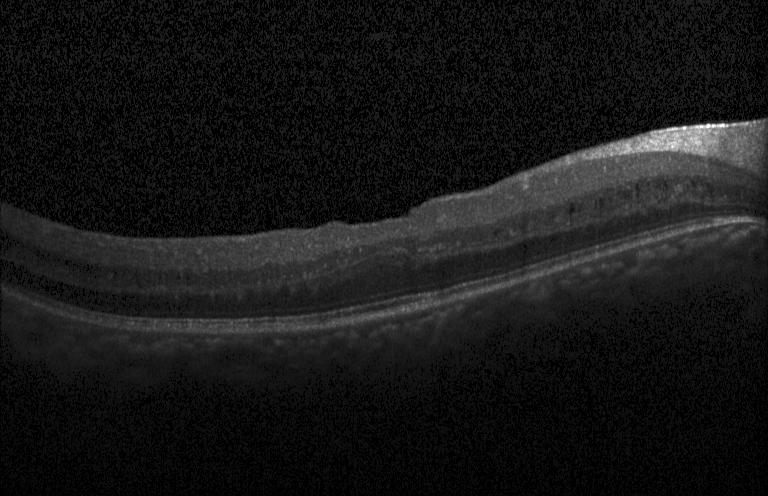

SD-OCT · horizontal scan through the fovea · optical coherence tomography scan. Assessment: diabetic macular edema.